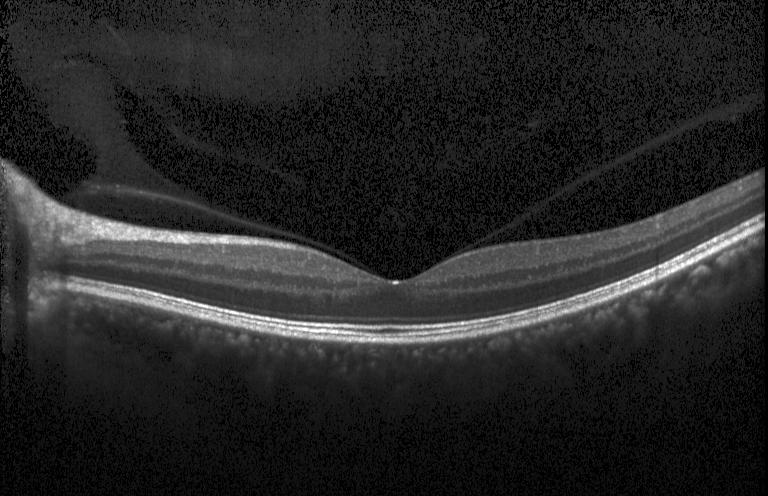

Macular scan, Heidelberg Spectralis, OCT line scan. OCT finding: no CNV, DME, or drusen.